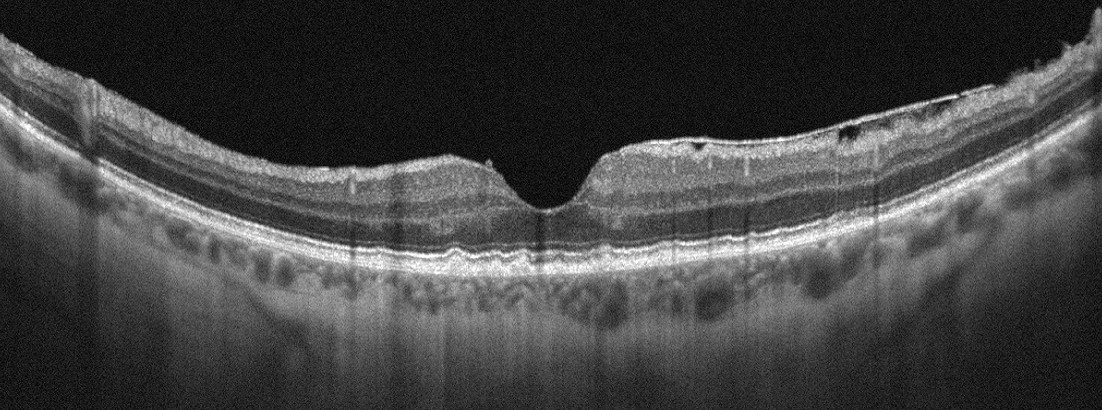

Instrument: Optovue Avanti RTVue XR; OCT B-scan; through the macula. OCT finding: epiretinal membrane (ERM).